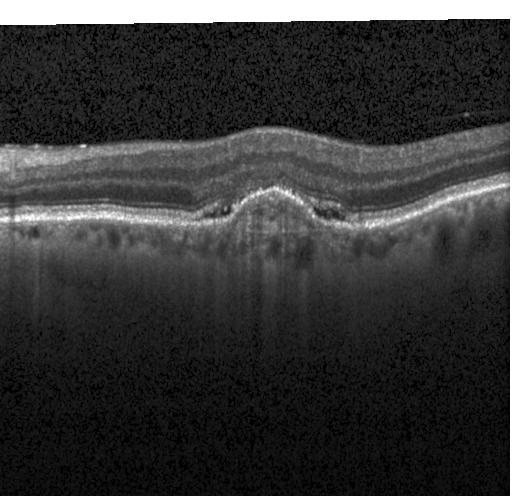

Retinal OCT cross-section showing choroidal neovascularization.